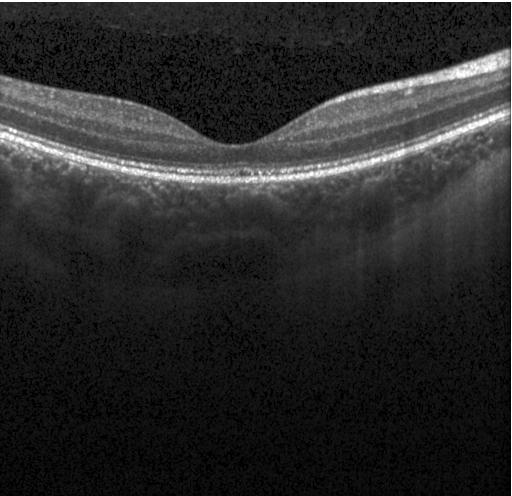

Retinal OCT B-scan. Spectral-domain OCT
Diagnosis: no choroidal neovascularization, no diabetic macular edema, and no drusen.